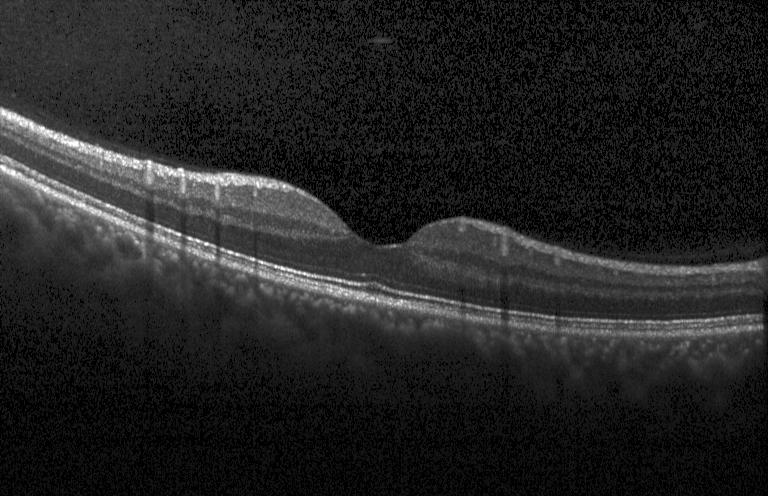 Through the macula, SD-OCT, Heidelberg Spectralis, OCT B-scan
Macular OCT: no evidence of CNV, DME, or drusen.